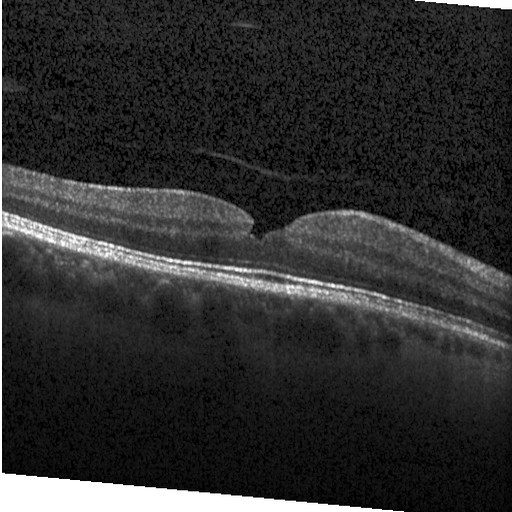 Through the macula · spectral-domain optical coherence tomography · Heidelberg Spectralis · retinal OCT B-scan — The scan shows diabetic macular edema.